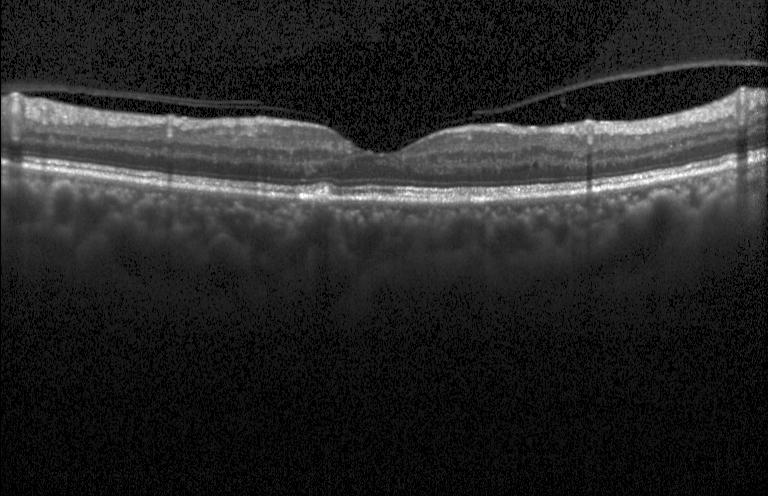 OCT line scan.
Impression: drusen.